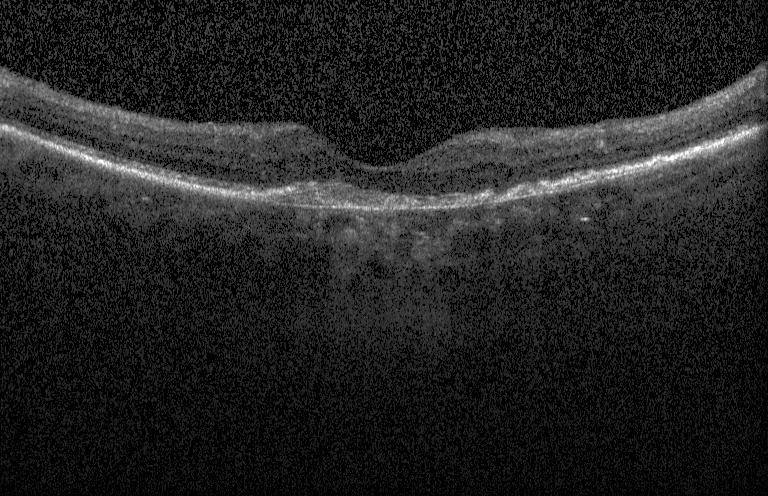

Finding: choroidal neovascularization.